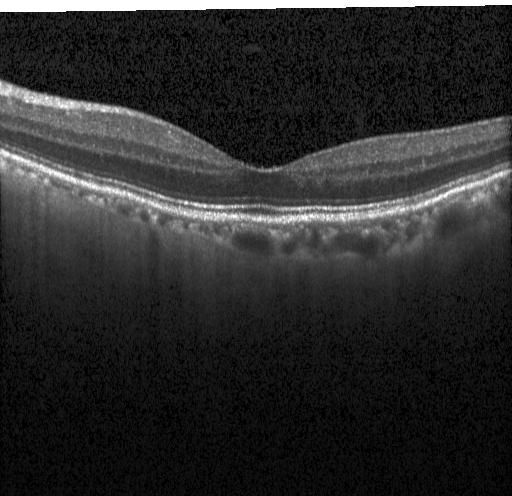
Diagnosis: no CNV, no DME, and no drusen.